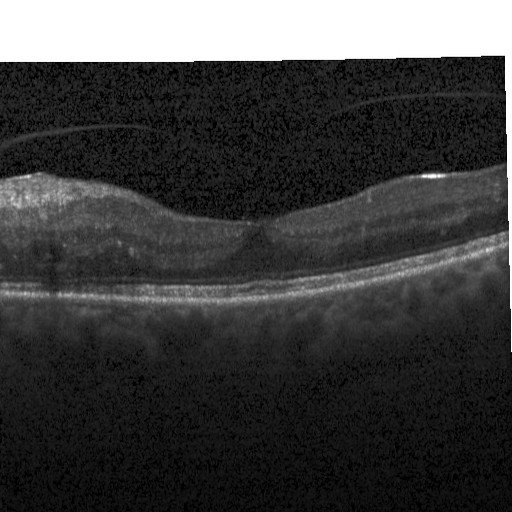

Optical coherence tomography B-scan — Impression: DME.